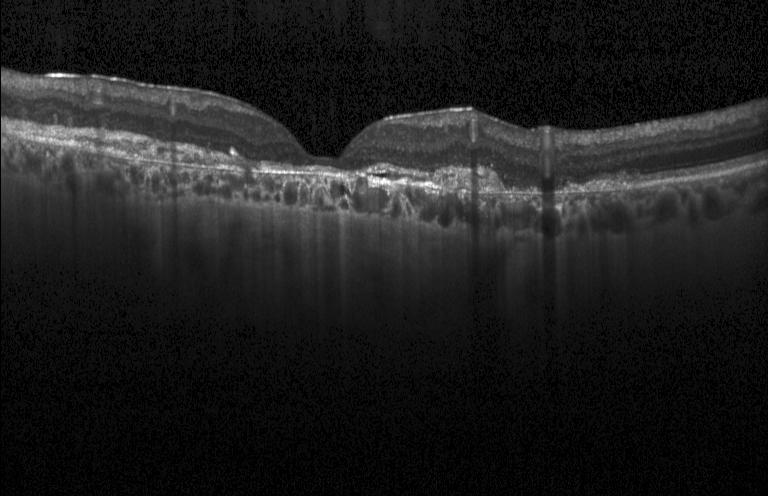 Dx: a choroidal neovascular membrane.